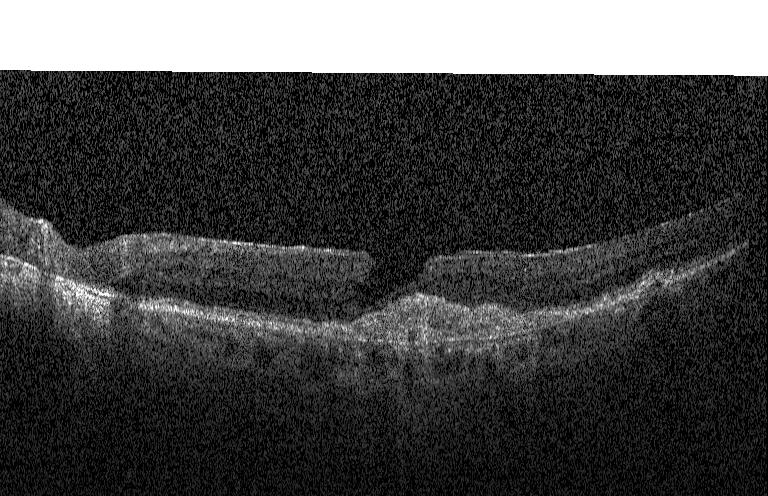

Dx: choroidal neovascularization.